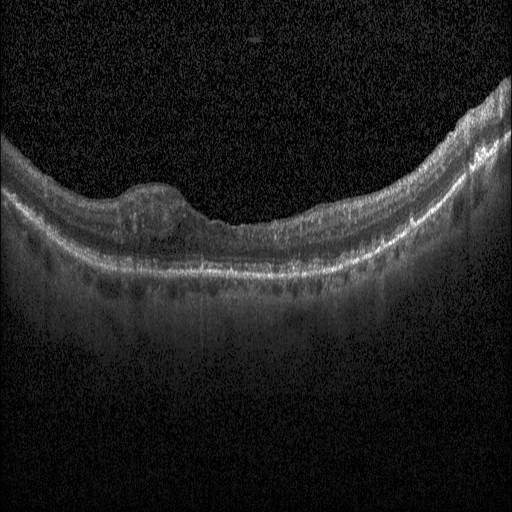 Macular scan, retinal OCT cross-section, acquired on a Heidelberg Spectralis, spectral-domain OCT
Diabetic macular edema (DME).